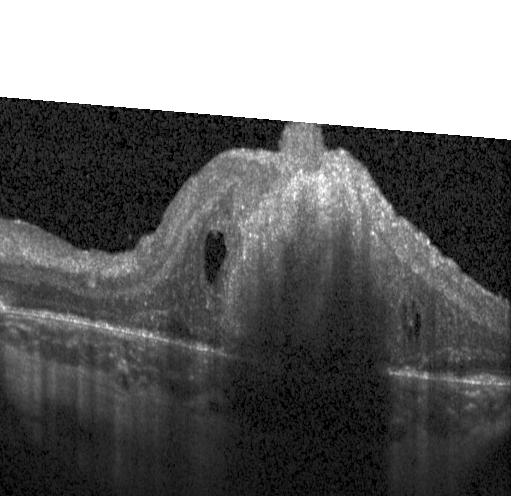 Instrument: Heidelberg Spectralis, through the macula, SD-OCT, retinal OCT B-scan
The scan shows CNV.